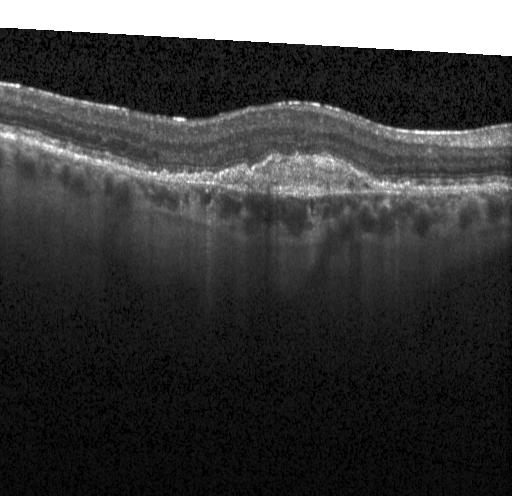

OCT finding: a choroidal neovascular membrane.